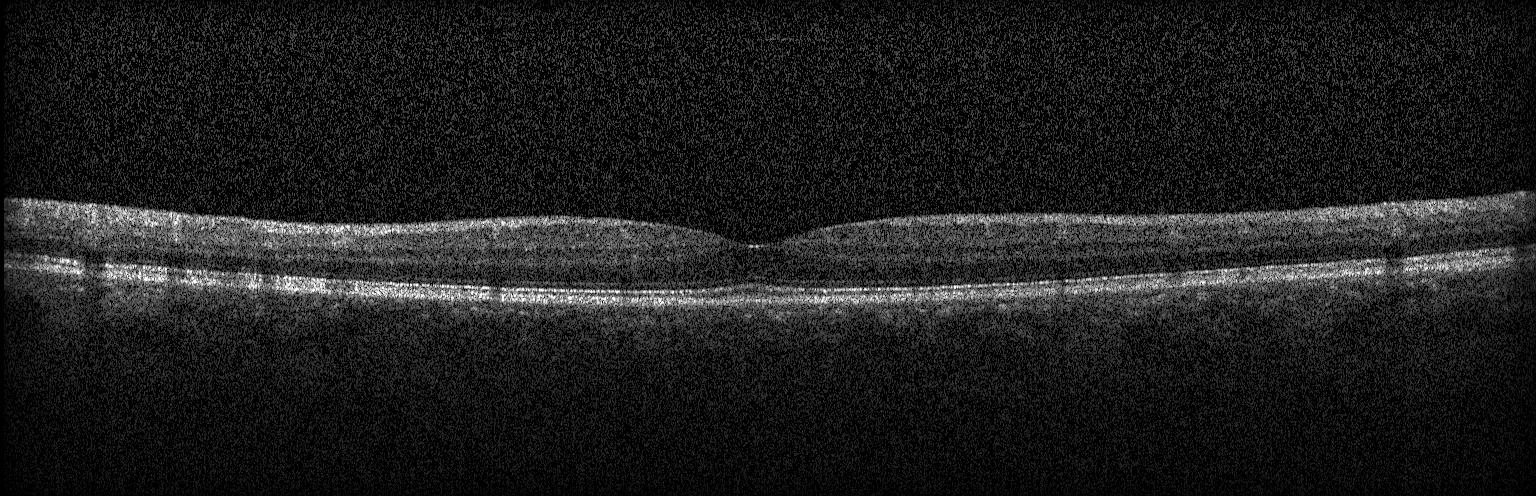 Macular OCT demonstrating no choroidal neovascularization, no diabetic macular edema, and no drusen.